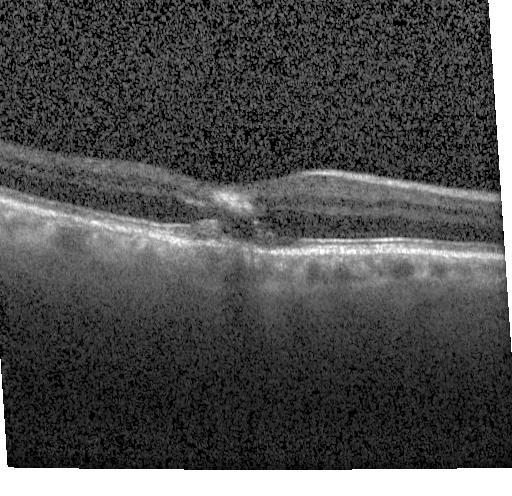

Retinal OCT cross-section — OCT finding: a choroidal neovascular membrane.